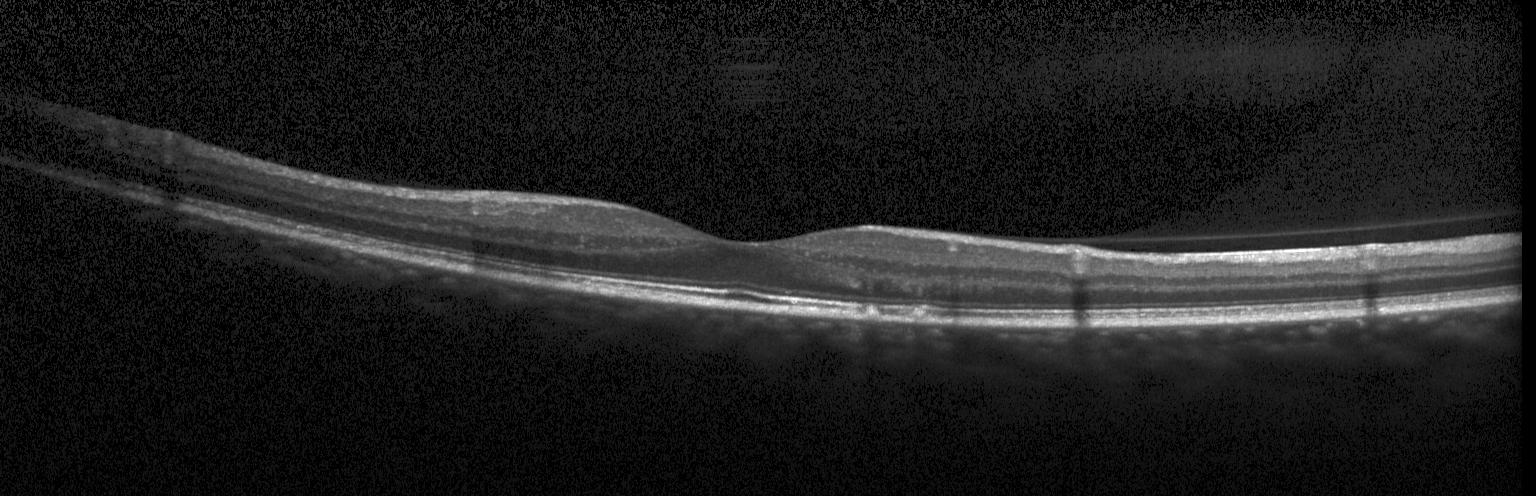
Optical coherence tomography scan
Macular OCT: multiple drusen.